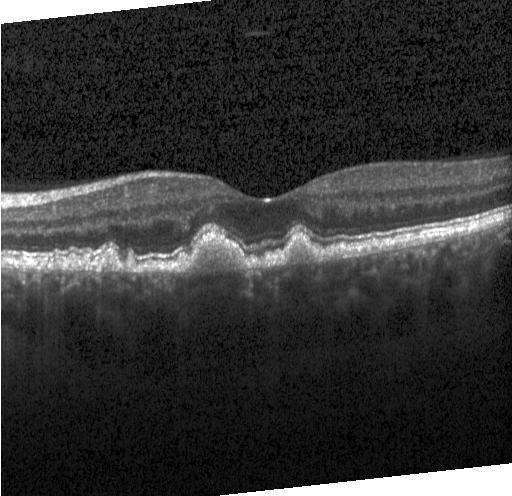 SD-OCT, OCT line scan
OCT finding: drusen.